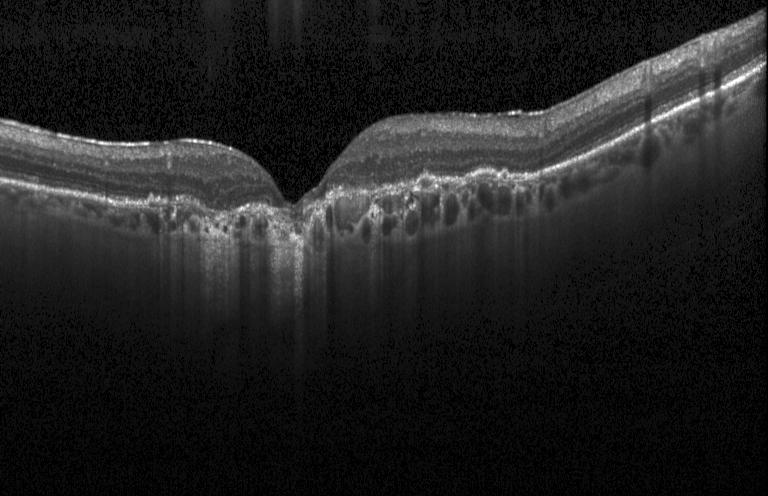

Spectral-domain OCT; OCT B-scan.
Finding: a choroidal neovascular membrane.